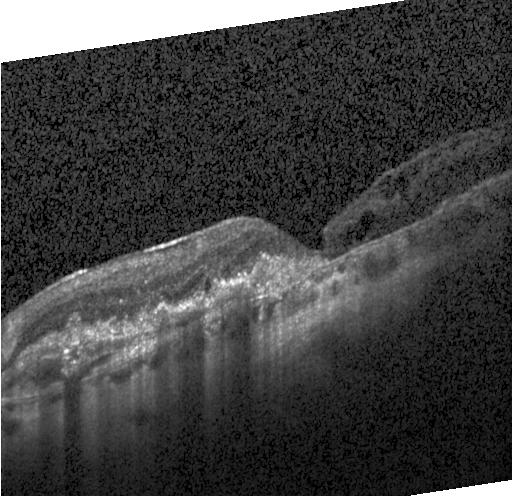 Choroidal neovascularization.